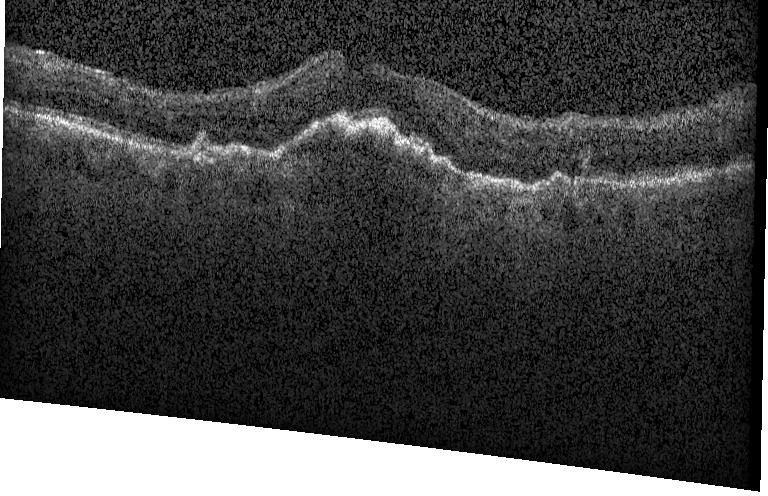 Retinal OCT B-scan; SD-OCT. Diagnosis: a choroidal neovascular membrane.